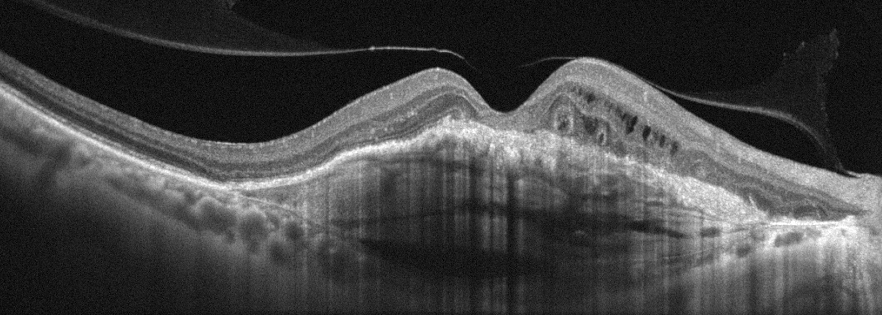 Oculus dexter; optical coherence tomography B-scan; macular scan; acquired on an Optovue Avanti RTVue XR — Impression: age-related macular degeneration (AMD).